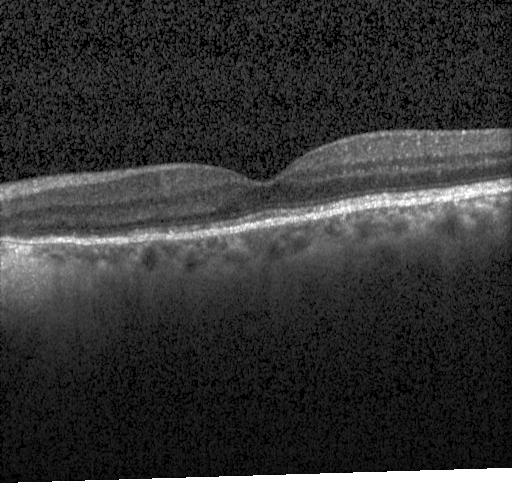
OCT B-scan. Instrument: Heidelberg Spectralis
Assessment: no choroidal neovascularization, no diabetic macular edema, and no drusen.